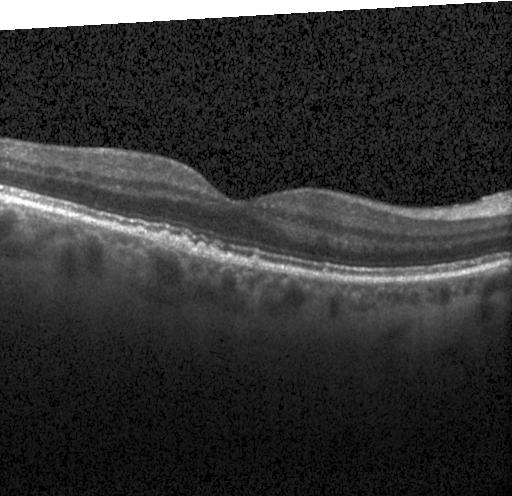
OCT B-scan — Finding: drusen.